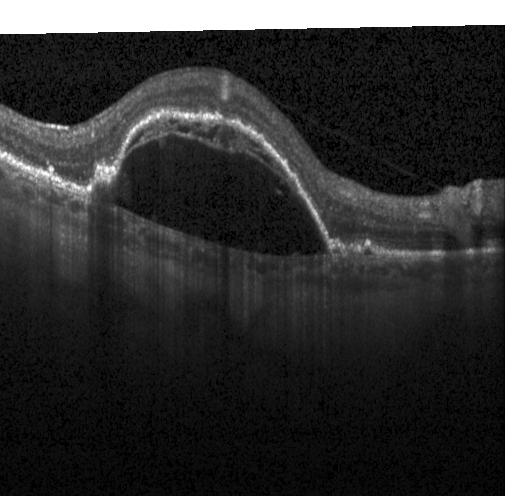 Spectral-domain OCT; acquired on a Heidelberg Spectralis; OCT line scan; macular scan — Assessment: choroidal neovascularization.